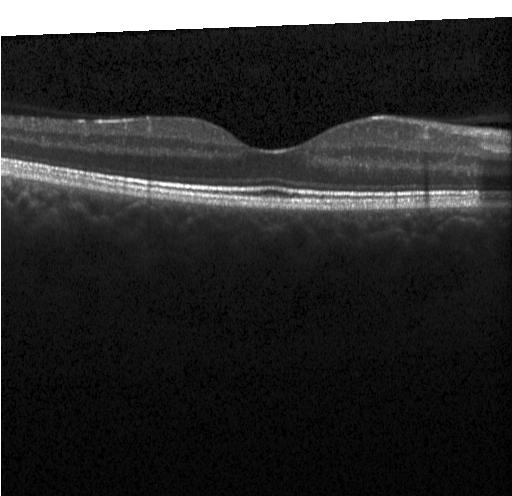 Dx: no choroidal neovascularization, no diabetic macular edema, and no drusen.